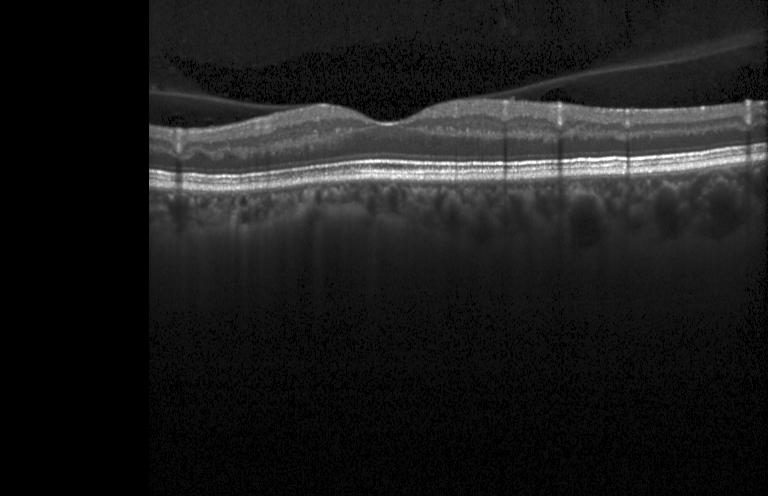

Dx: no choroidal neovascularization, diabetic macular edema, or drusen.